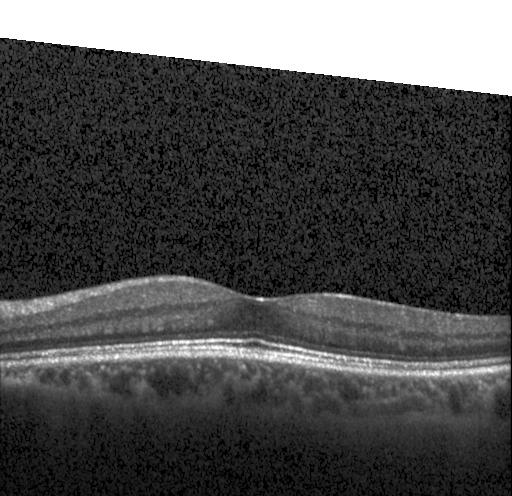 OCT scan showing no choroidal neovascularization, no diabetic macular edema, and no drusen.